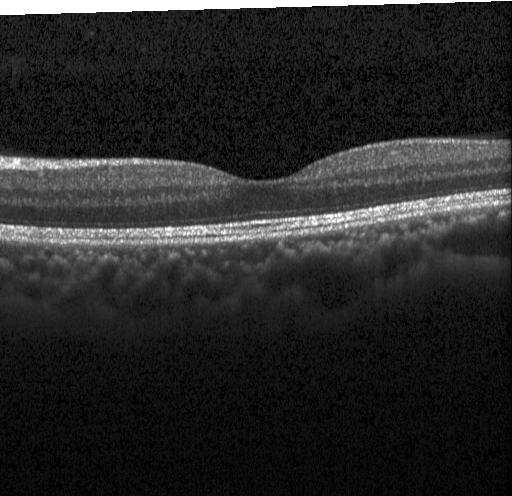 Fovea-centered. SD-OCT. Heidelberg Spectralis OCT system. Optical coherence tomography B-scan
Diagnosis: no evidence of choroidal neovascularization, diabetic macular edema, or drusen.